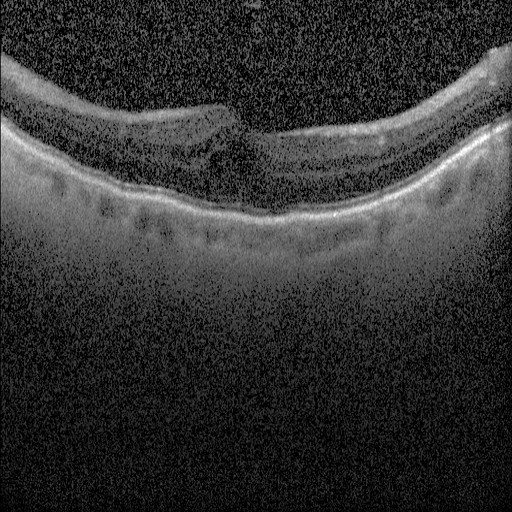

Acquired on a Heidelberg Spectralis. Retinal OCT B-scan. Spectral-domain OCT.
Macular OCT: DME.